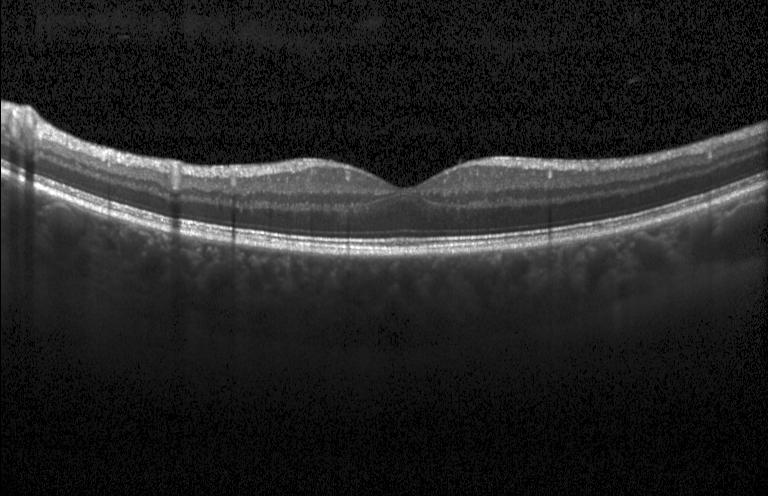
Through the macula · retinal OCT cross-section · acquired on a Heidelberg Spectralis.
Finding: no evidence of choroidal neovascularization, diabetic macular edema, or drusen.